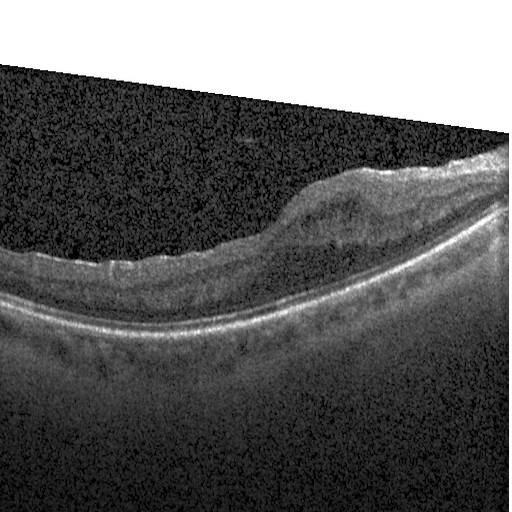

Macular scan; retinal OCT cross-section; instrument: Heidelberg Spectralis; spectral-domain optical coherence tomography — Diagnosis: diabetic macular edema (DME).